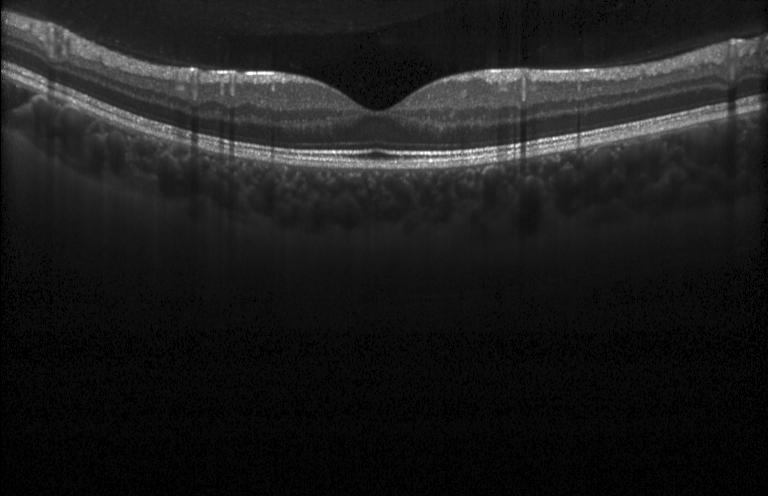
OCT scan showing no CNV, DME, or drusen.